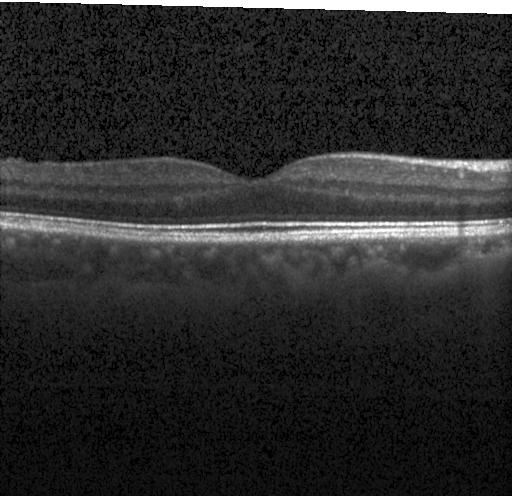
Finding: neither CNV, DME, nor drusen.